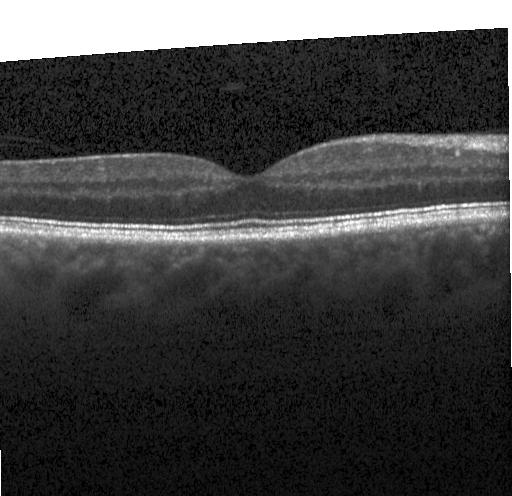
Spectral-domain OCT. Optical coherence tomography scan. Diagnosis: no choroidal neovascularization, no diabetic macular edema, and no drusen.